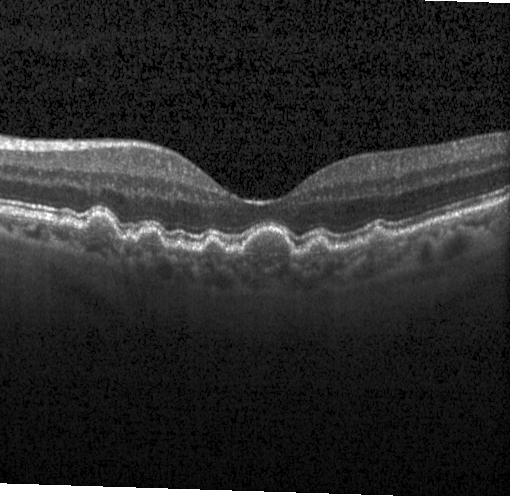 Diagnosis: sub-RPE drusenoid deposits.